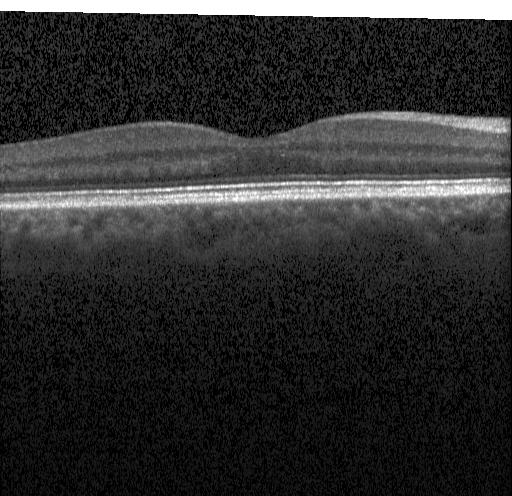
Heidelberg Spectralis OCT system. OCT B-scan. Centered on the fovea. SD-OCT.
No choroidal neovascularization, no diabetic macular edema, and no drusen.